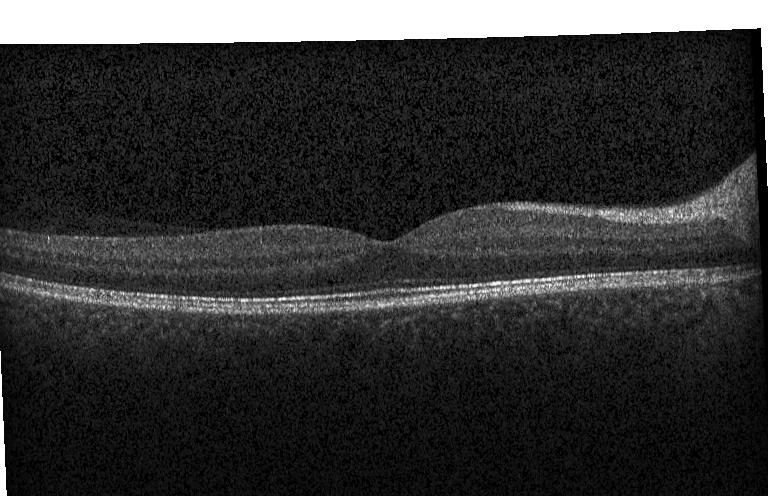 Heidelberg Spectralis; spectral-domain optical coherence tomography; fovea-centered; retinal OCT cross-section — Impression: neither choroidal neovascularization, diabetic macular edema, nor drusen.